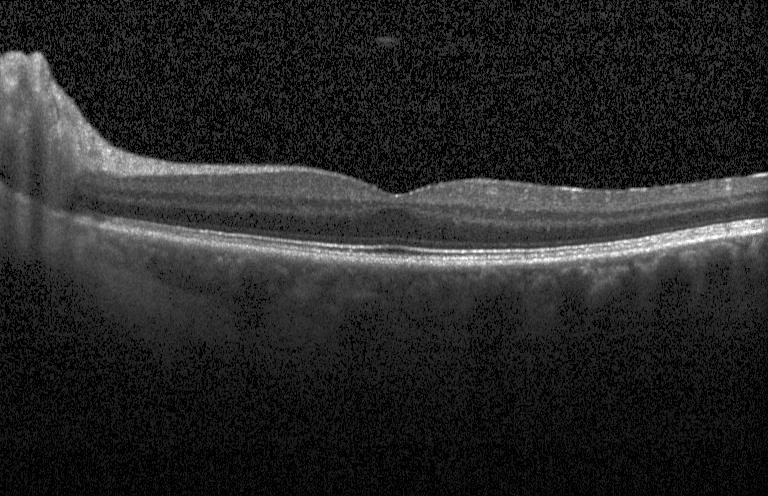
Spectral-domain optical coherence tomography; OCT B-scan.
OCT finding: neither choroidal neovascularization, diabetic macular edema, nor drusen.